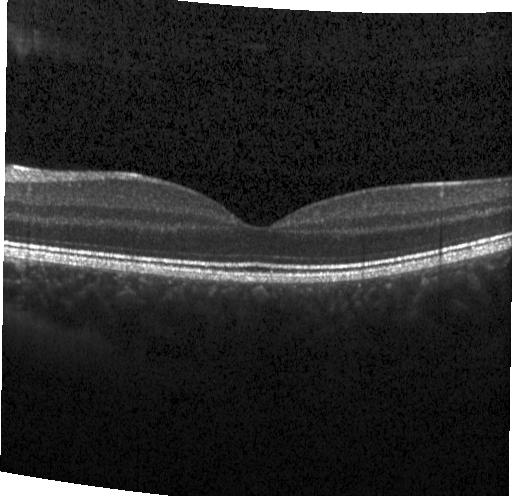
Optical coherence tomography scan.
Finding: no evidence of CNV, DME, or drusen.